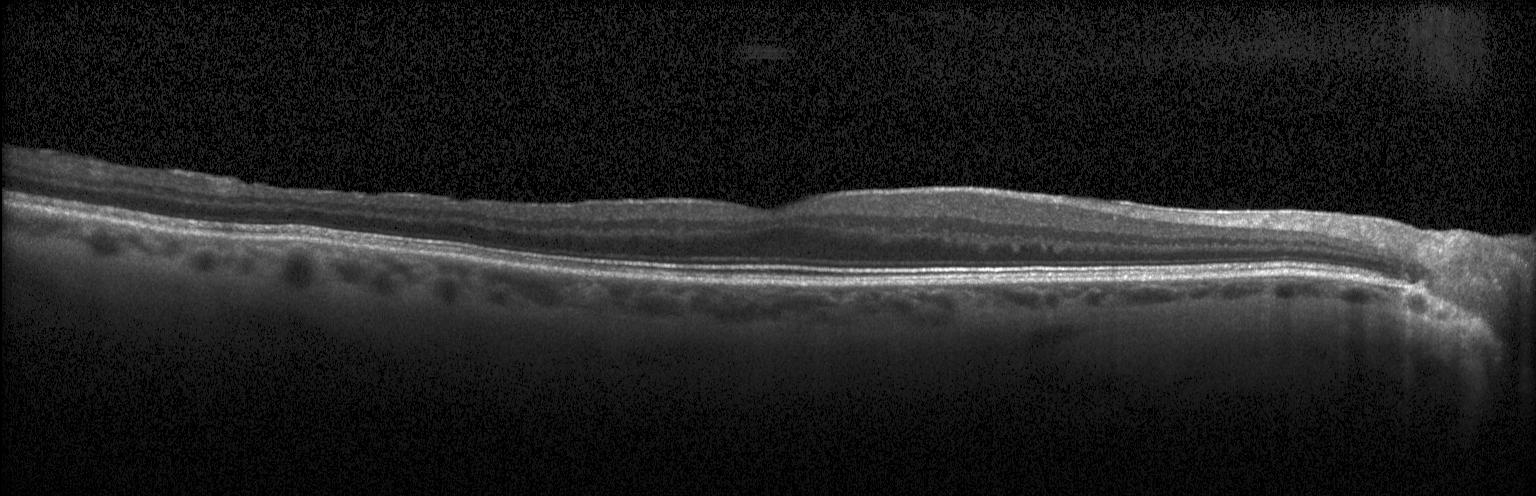
Centered on the fovea · optical coherence tomography scan
This B-scan demonstrates no CNV, no DME, and no drusen.